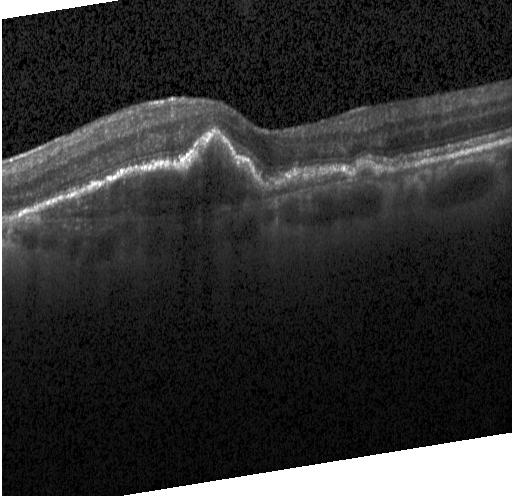

Heidelberg Spectralis, spectral-domain OCT, optical coherence tomography B-scan, centered on the fovea — Diagnosis: a choroidal neovascular membrane.